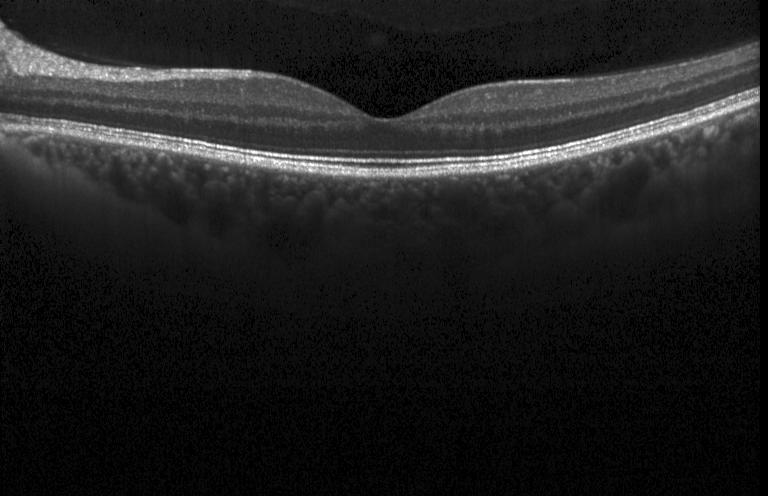
Horizontal scan through the fovea · optical coherence tomography scan · instrument: Heidelberg Spectralis — Dx: no evidence of choroidal neovascularization, diabetic macular edema, or drusen.